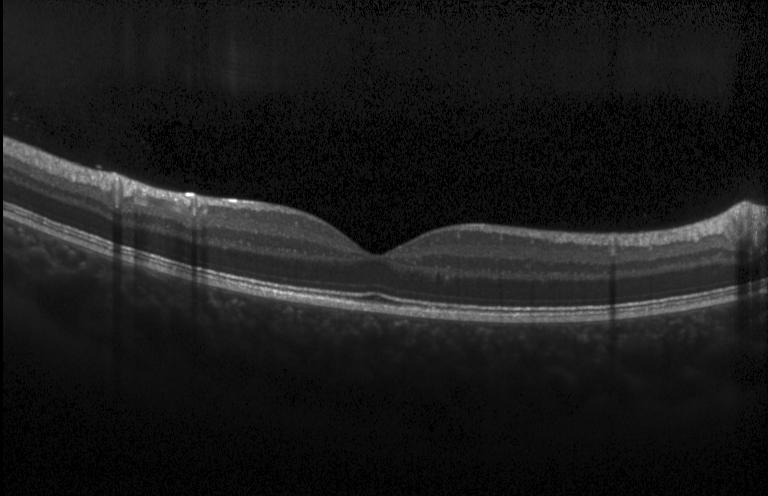
Spectral-domain OCT B-scan: no evidence of choroidal neovascularization, diabetic macular edema, or drusen.